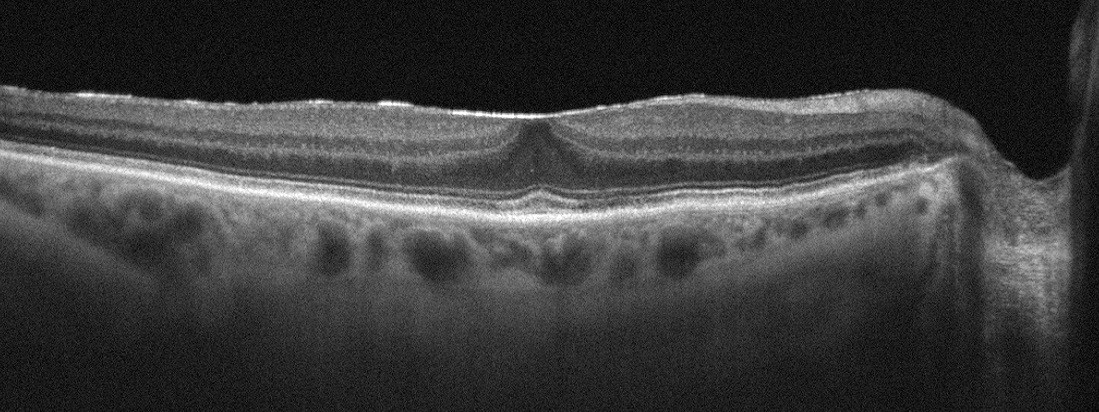

Macular scan; optical coherence tomography B-scan; acquired on an Optovue Avanti RTVue XR.
Epiretinal membrane.